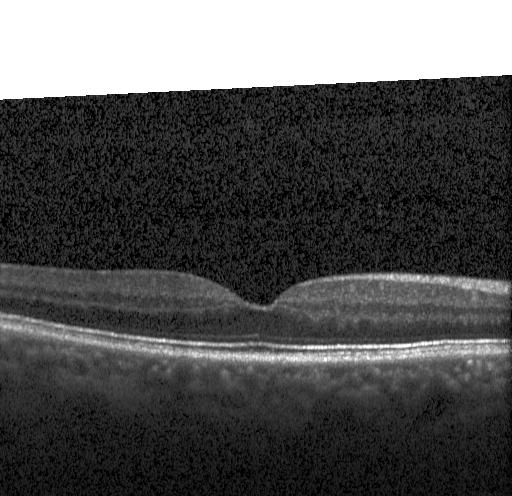

Assessment: neither choroidal neovascularization, diabetic macular edema, nor drusen.